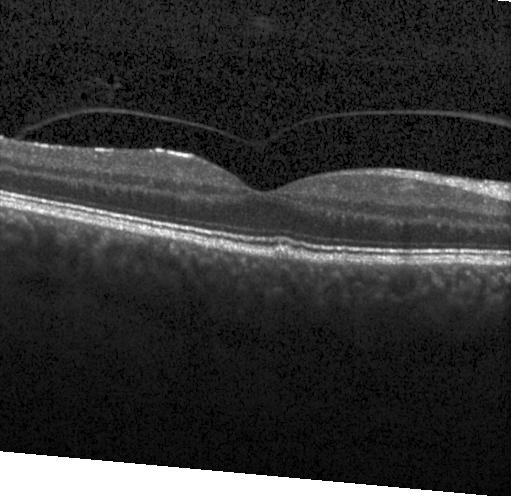
Through the macula · retinal OCT cross-section
Finding: sub-RPE drusenoid deposits.